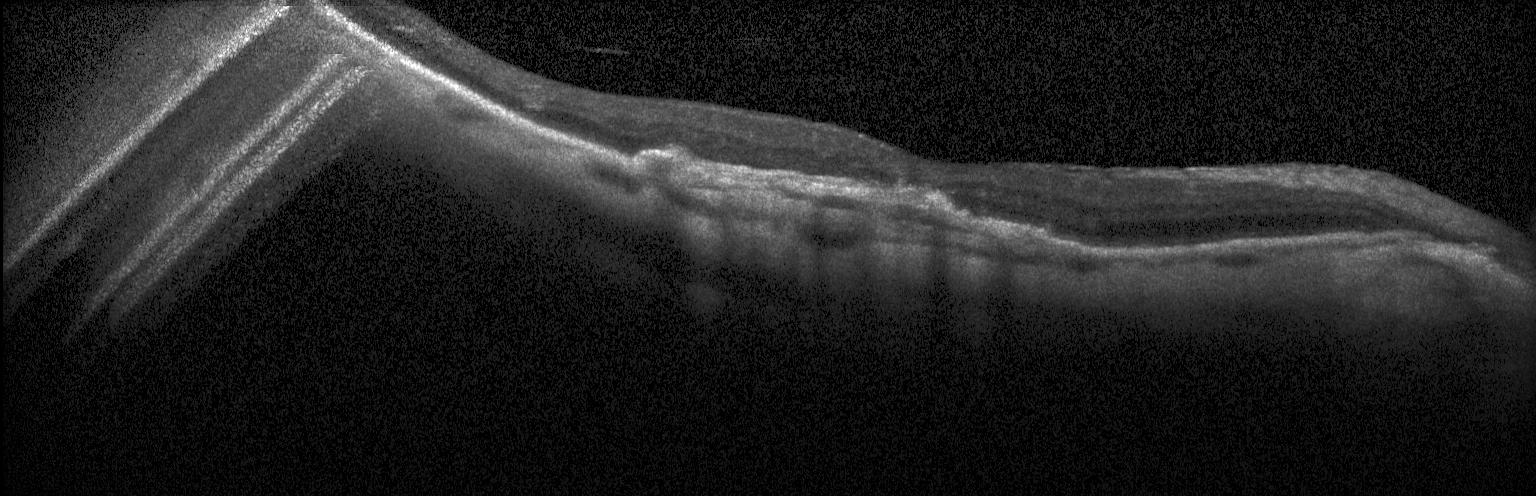

Diagnosis: a choroidal neovascular membrane.